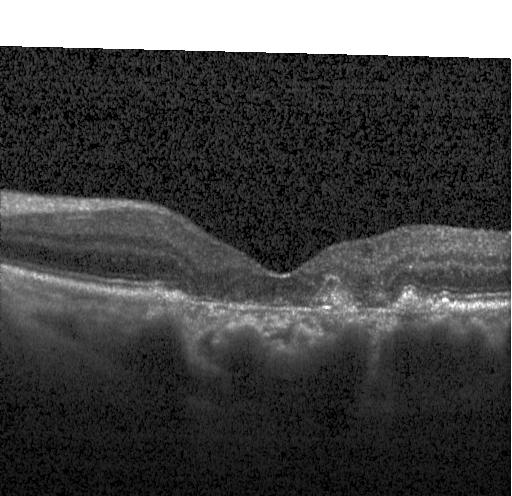 Assessment: CNV.